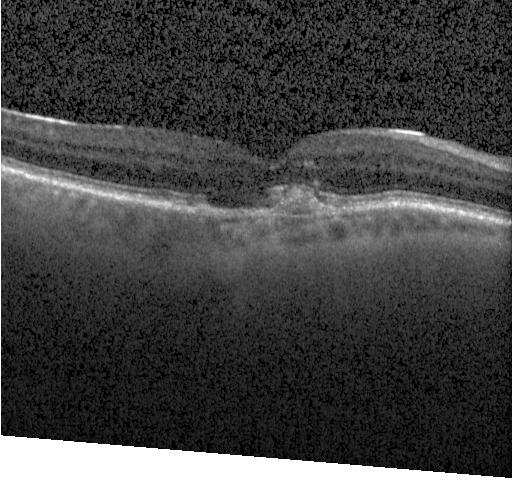

Spectral-domain optical coherence tomography. Retinal OCT B-scan. Acquired on a Heidelberg Spectralis
A choroidal neovascular membrane.